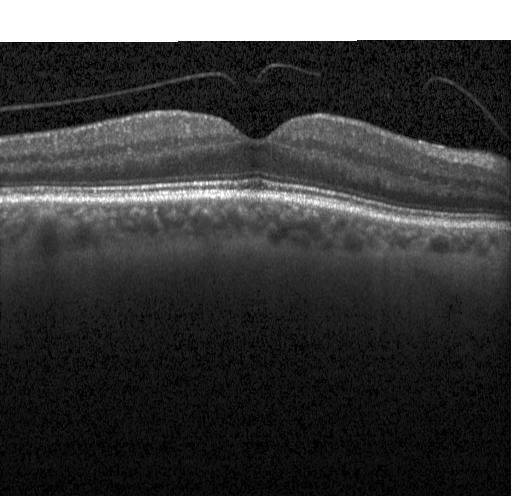
Centered on the fovea · optical coherence tomography B-scan.
Macular OCT: no CNV, no DME, and no drusen.